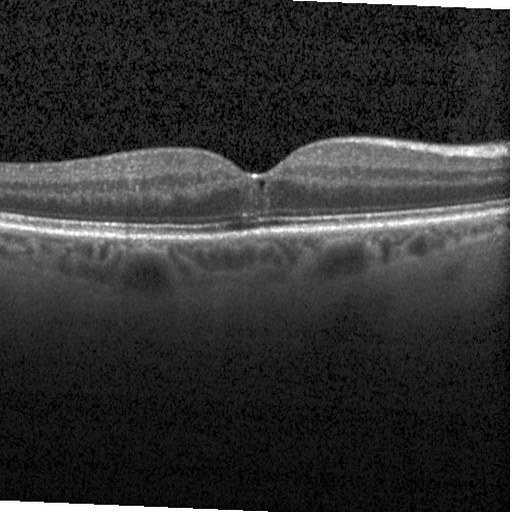

Finding: DME.